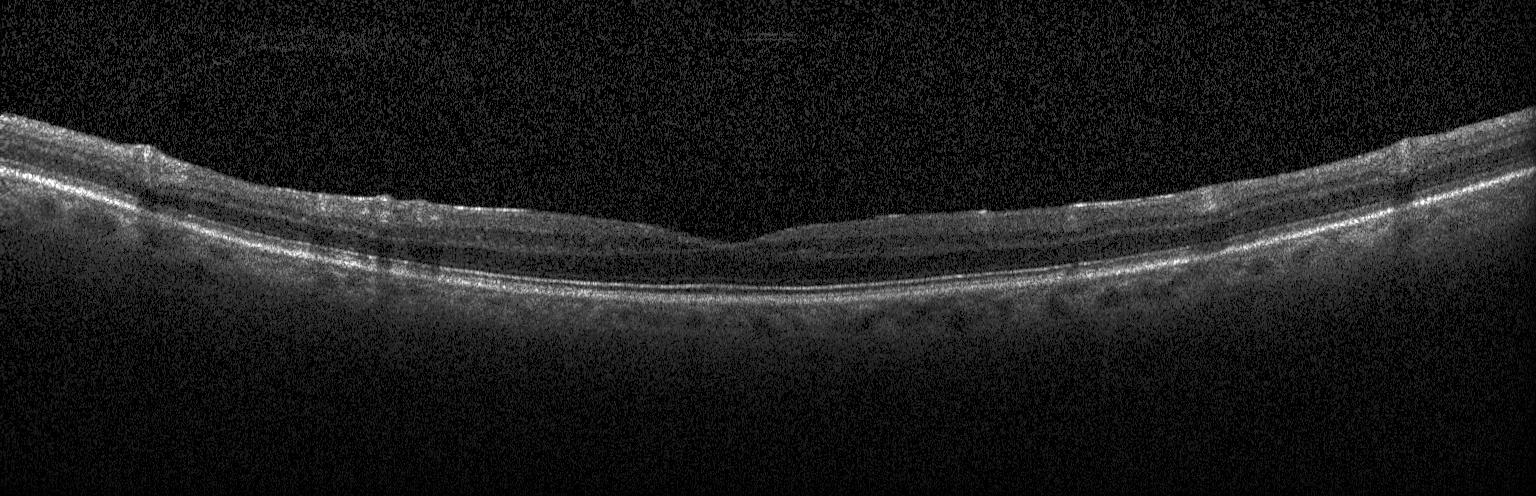 Optical coherence tomography B-scan.
The scan shows no evidence of CNV, DME, or drusen.